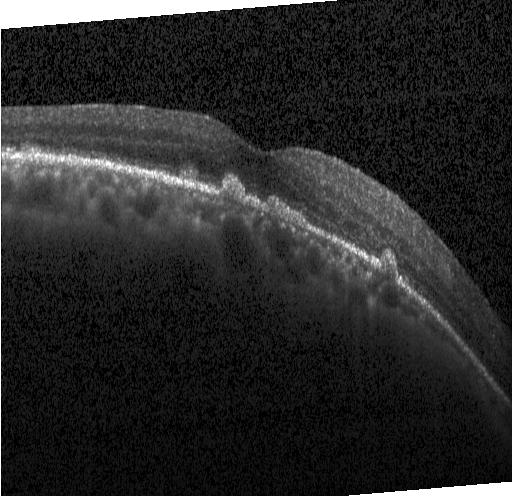
OCT scan showing sub-RPE drusenoid deposits.